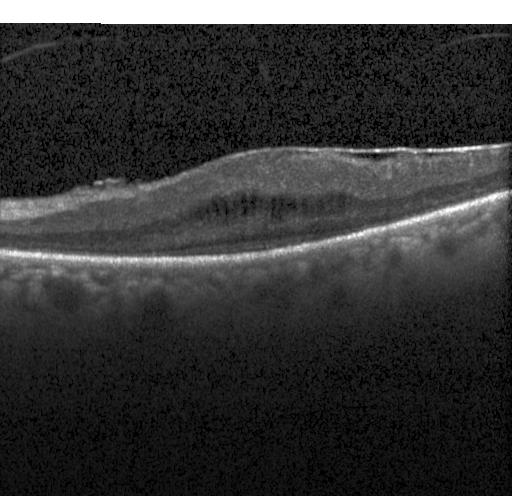 Diagnosis: diabetic macular edema (DME).